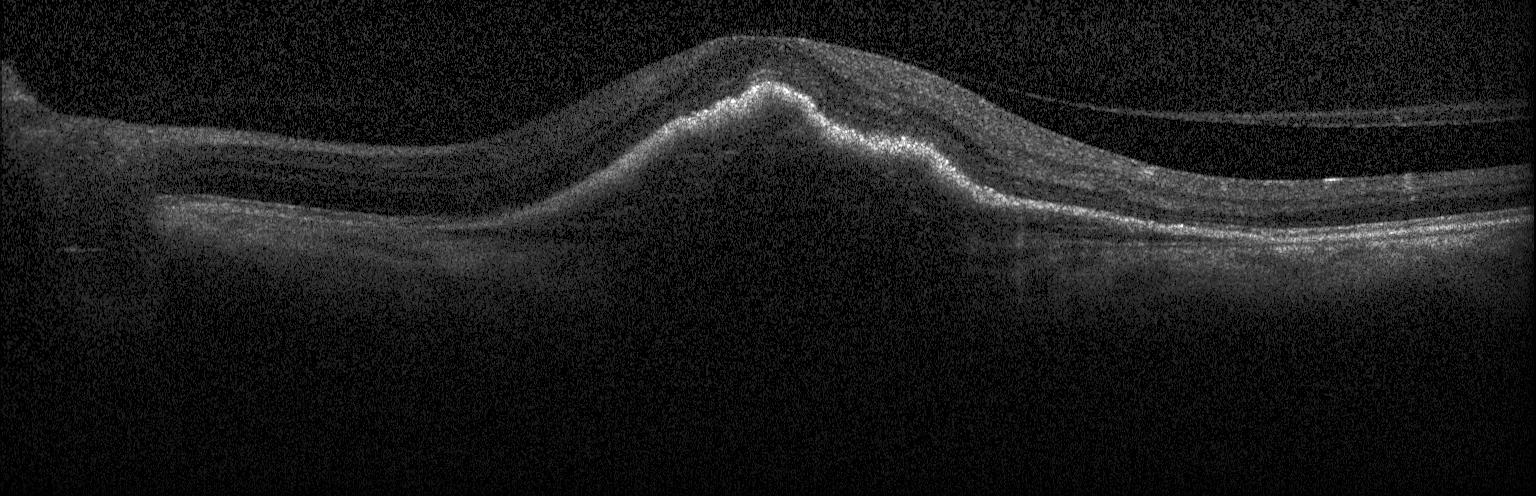

OCT finding: choroidal neovascularization.